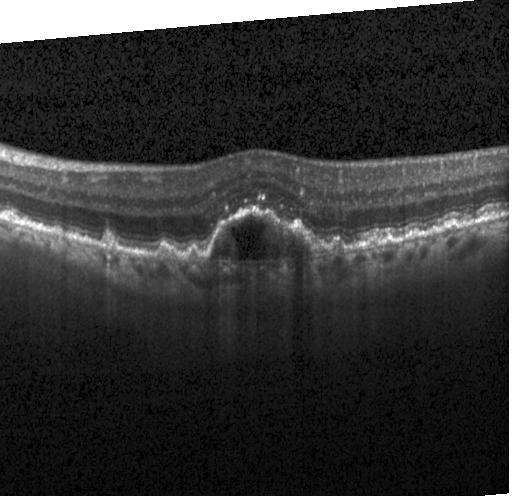

Through the macula. OCT line scan. Macular OCT: a choroidal neovascular membrane.